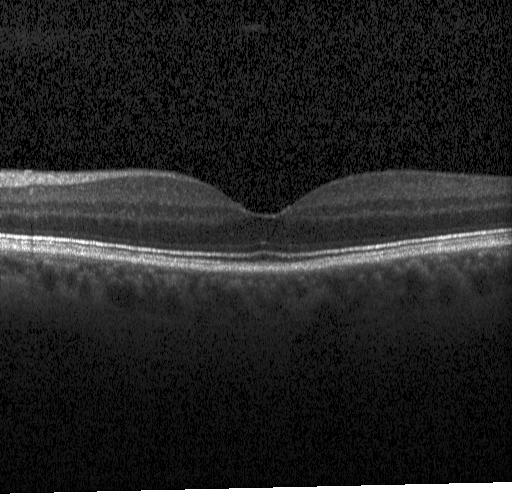
OCT B-scan showing no CNV, DME, or drusen.